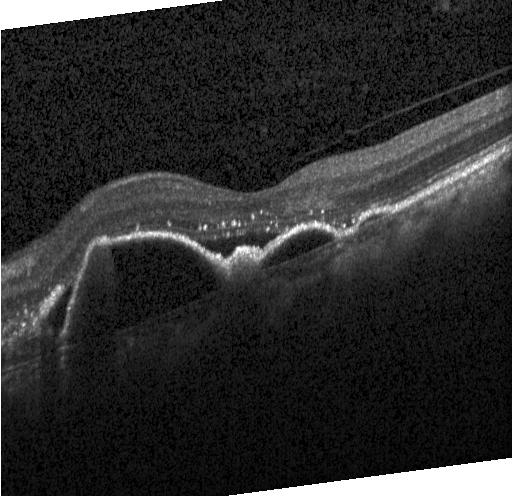

Diagnosis: a choroidal neovascular membrane.